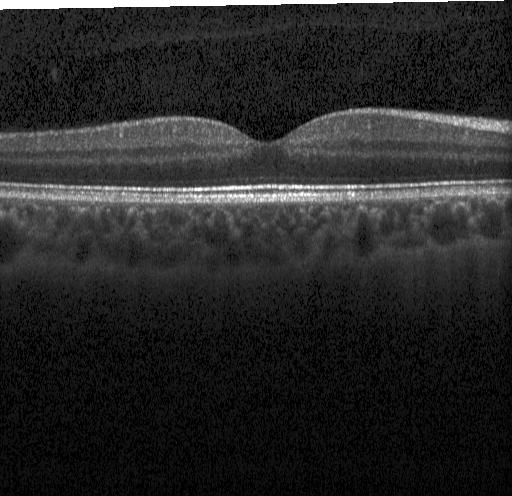 OCT B-scan, SD-OCT, horizontal scan through the fovea, Heidelberg Spectralis. Impression: no evidence of choroidal neovascularization, diabetic macular edema, or drusen.